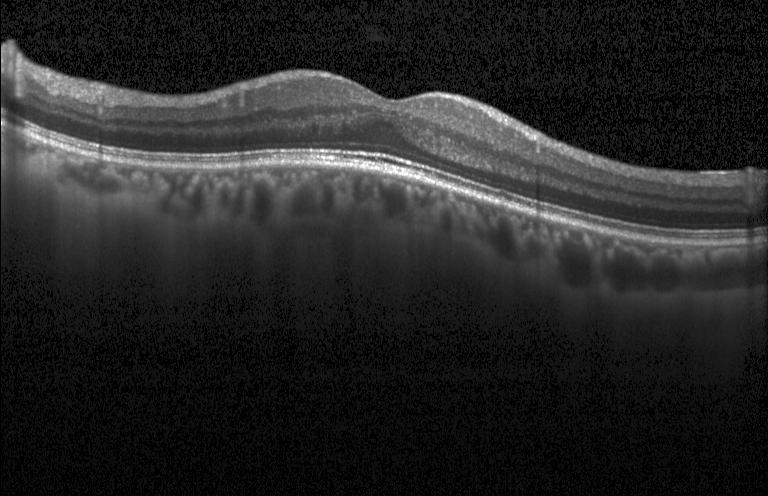

Spectral-domain OCT. Through the macula. Heidelberg Spectralis OCT system. Optical coherence tomography B-scan — Finding: no choroidal neovascularization, diabetic macular edema, or drusen.